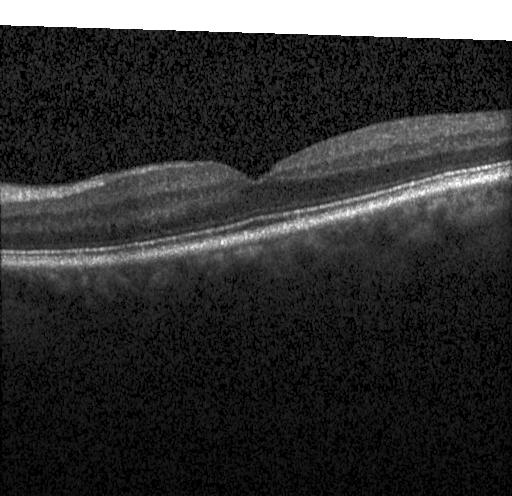
Acquired on a Heidelberg Spectralis. Fovea-centered. Spectral-domain OCT. Optical coherence tomography scan. The scan shows no choroidal neovascularization, no diabetic macular edema, and no drusen.